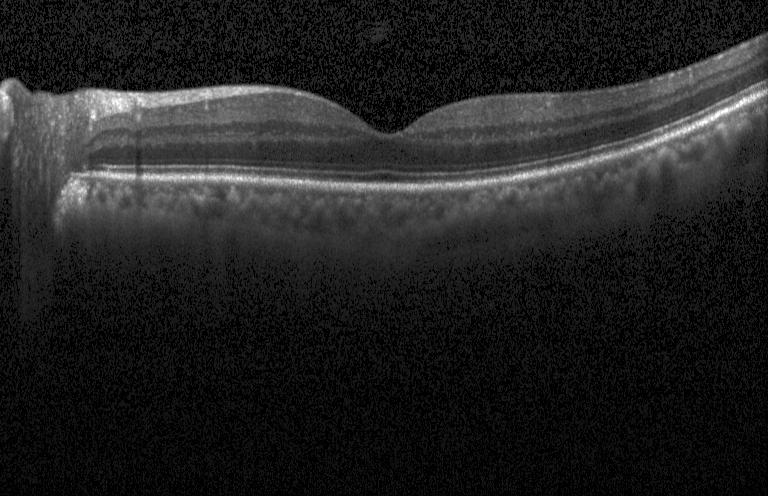

Diagnosis: no evidence of CNV, DME, or drusen.